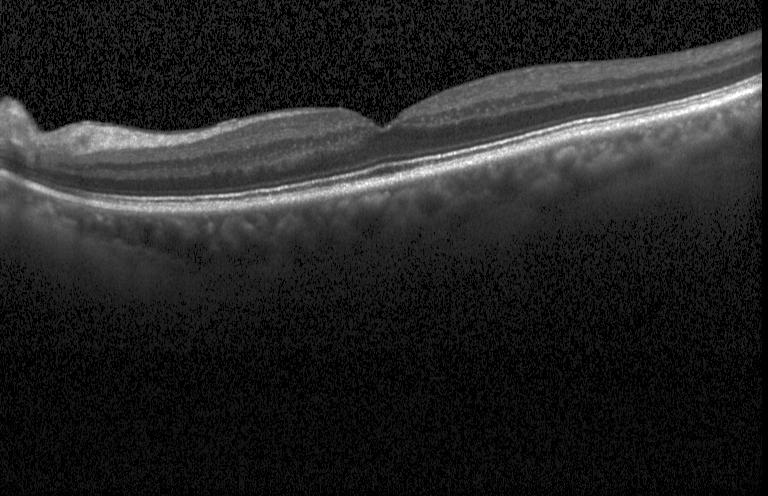

Finding: no CNV, DME, or drusen.